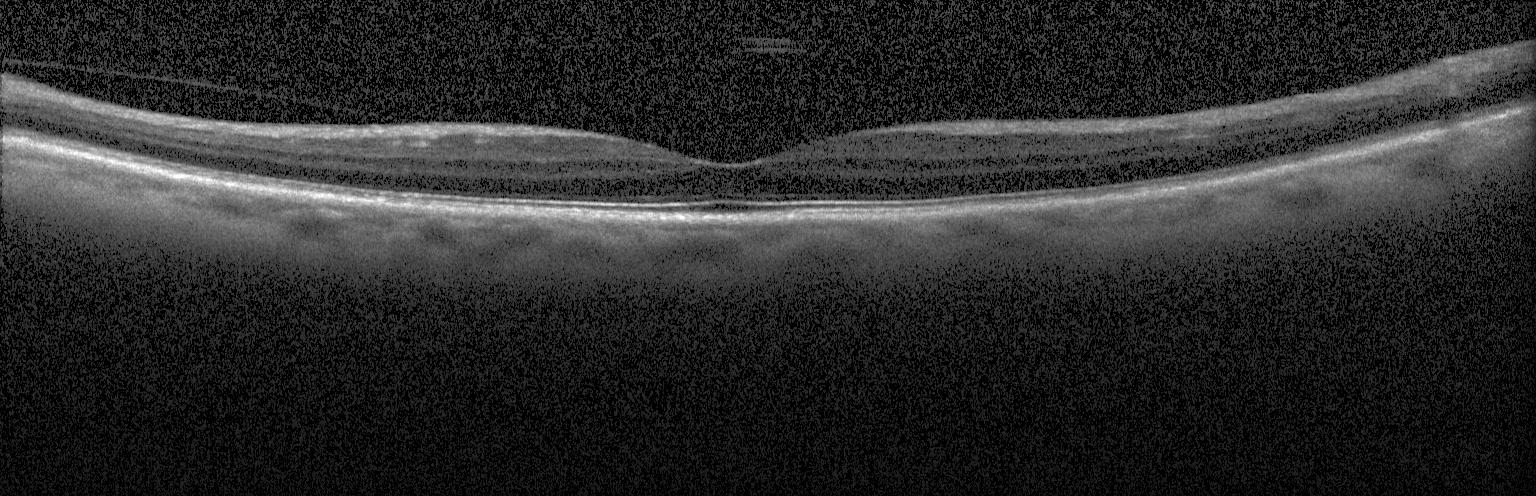

Finding: neither choroidal neovascularization, diabetic macular edema, nor drusen.